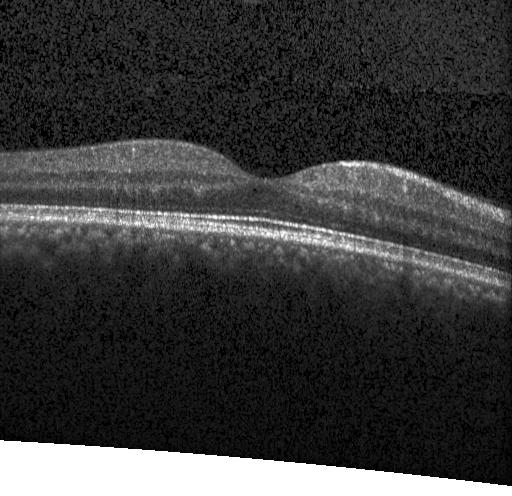
OCT line scan; Heidelberg Spectralis.
This B-scan demonstrates neither CNV, DME, nor drusen.